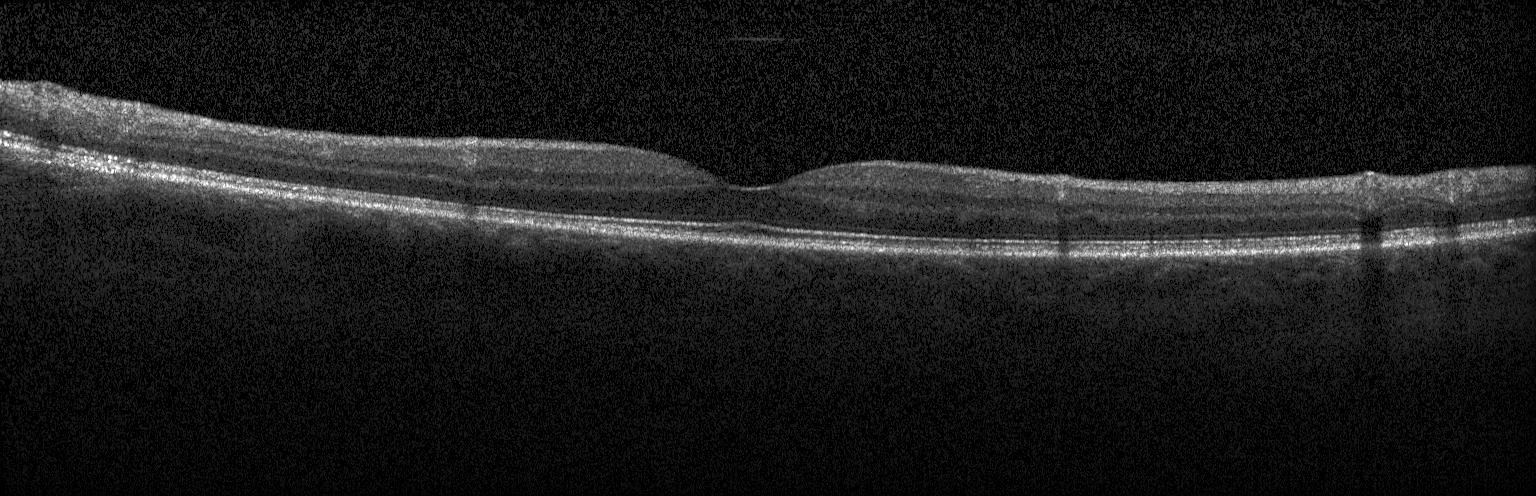

Optical coherence tomography scan.
Assessment: no evidence of choroidal neovascularization, diabetic macular edema, or drusen.